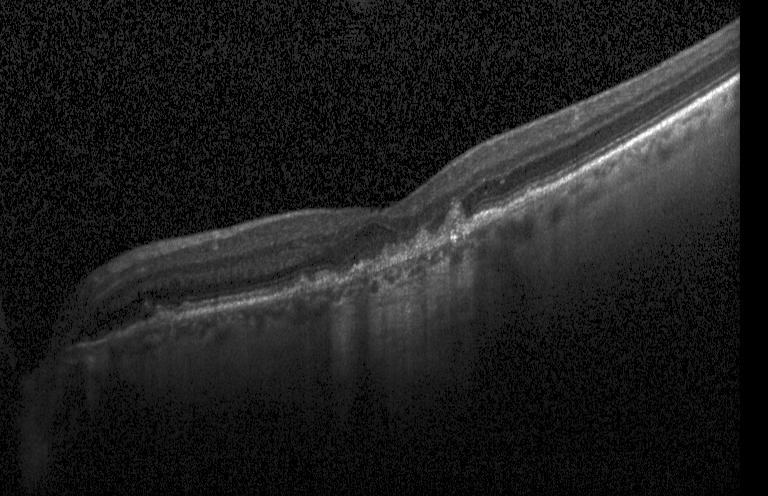

Finding: choroidal neovascularization.